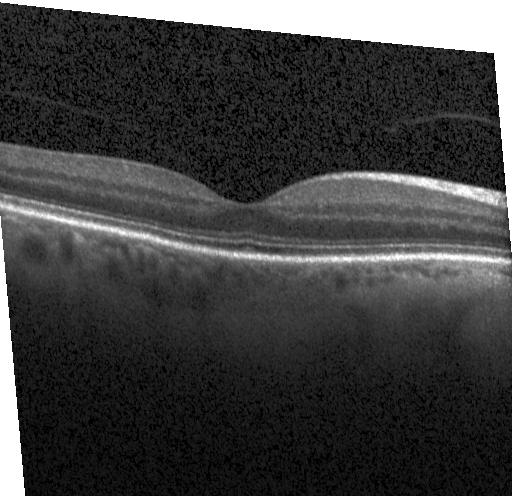

Diagnosis: no CNV, no DME, and no drusen.